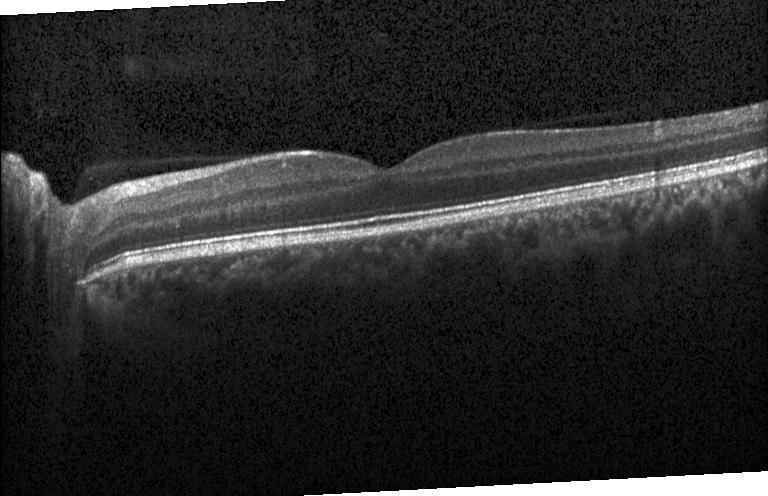

Neither choroidal neovascularization, diabetic macular edema, nor drusen.